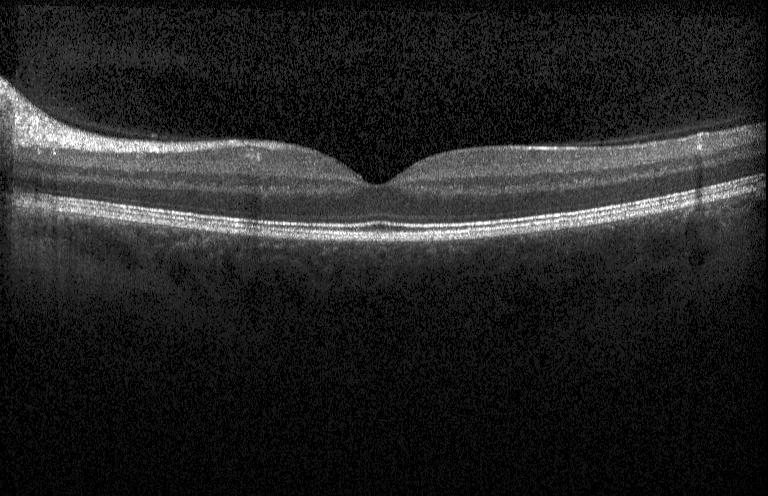

Macular OCT demonstrating no evidence of CNV, DME, or drusen.